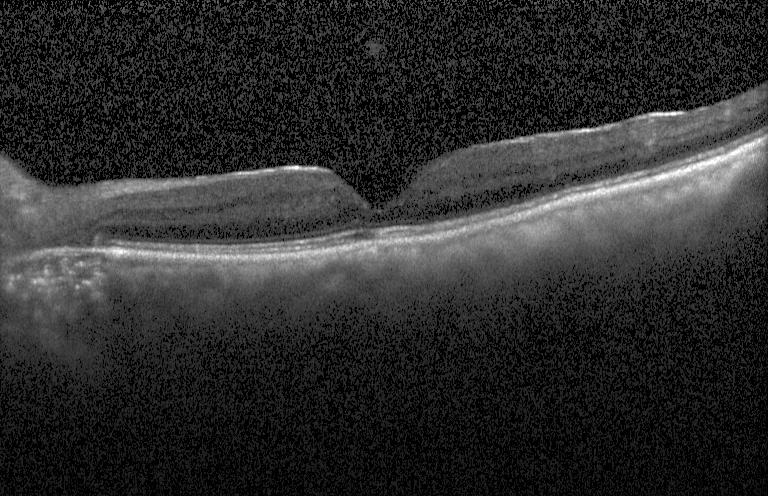 Acquired on a Heidelberg Spectralis. Spectral-domain OCT. Retinal OCT cross-section. Horizontal scan through the fovea — Diagnosis: no CNV, DME, or drusen.